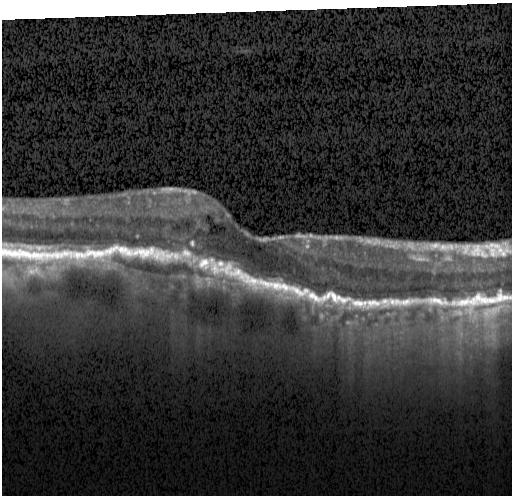 SD-OCT · retinal OCT cross-section · acquired on a Heidelberg Spectralis · centered on the fovea
Finding: a choroidal neovascular membrane.